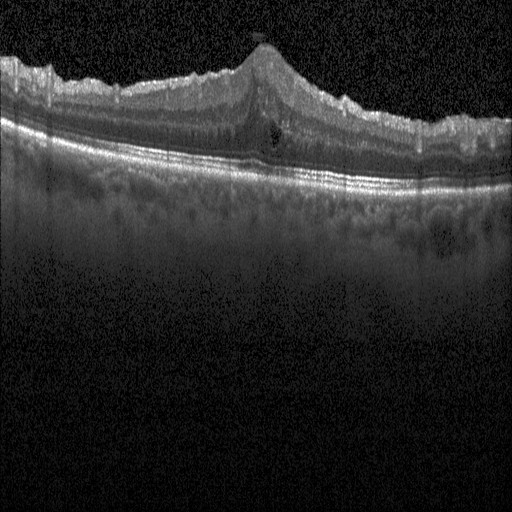

Finding: diabetic macular edema.